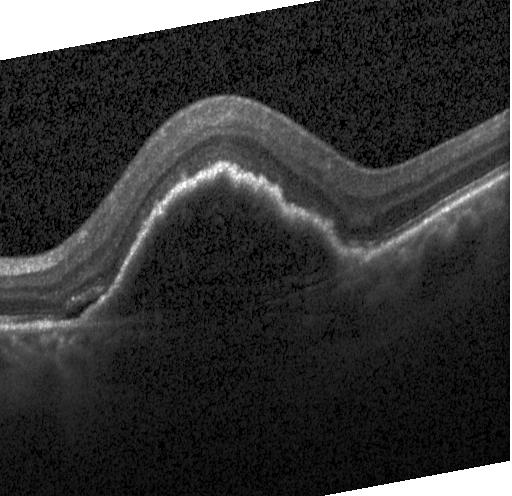
Retinal OCT cross-section, spectral-domain OCT — Impression: CNV.